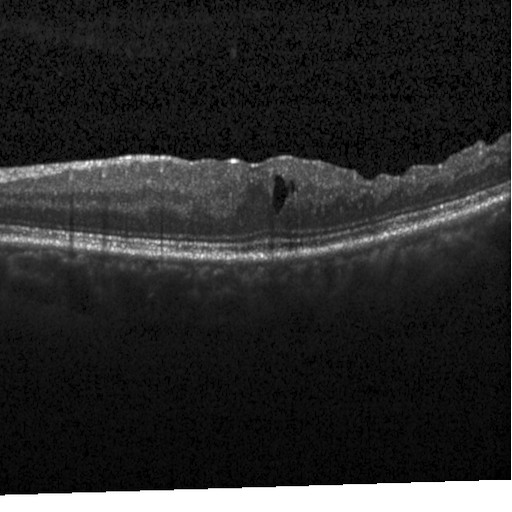 Through the macula. SD-OCT. Acquired on a Heidelberg Spectralis. OCT line scan
Diabetic macular edema (DME).